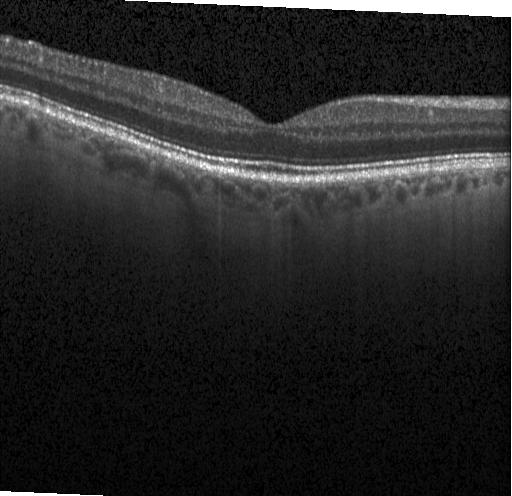 Finding: no CNV, DME, or drusen.